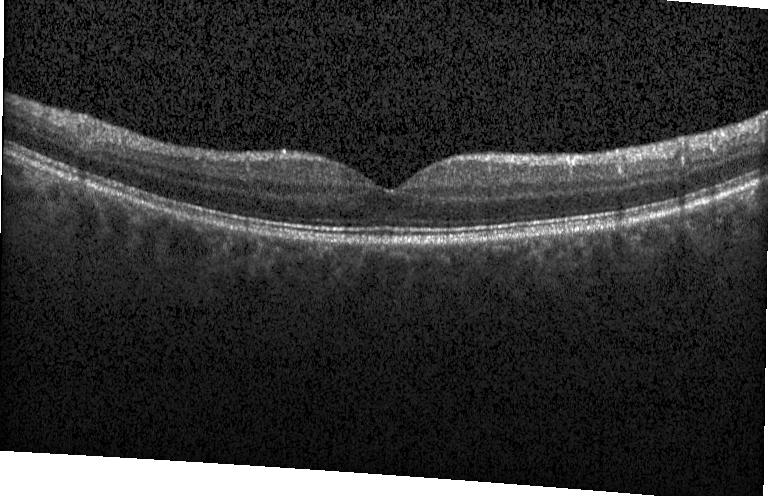
Optical coherence tomography B-scan · horizontal scan through the fovea — Impression: no choroidal neovascularization, diabetic macular edema, or drusen.